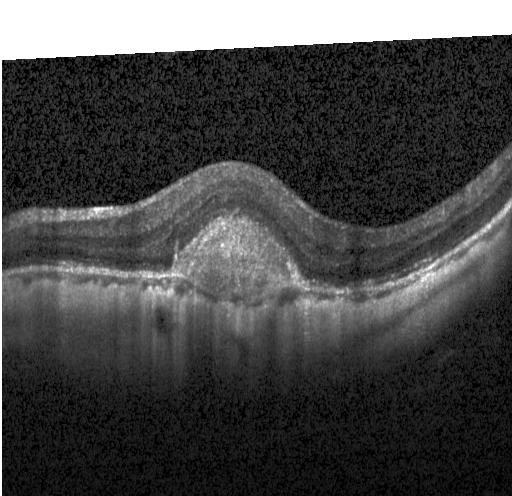

OCT finding: a choroidal neovascular membrane.